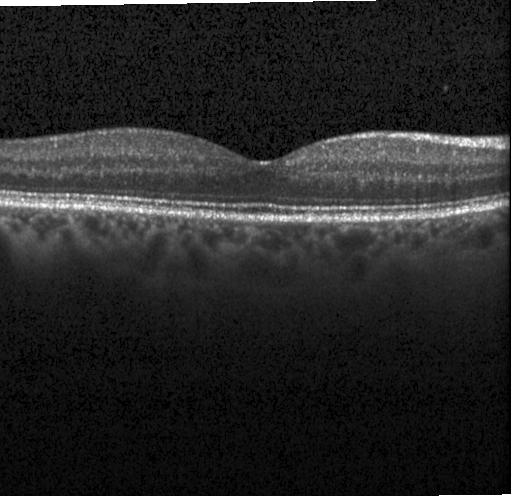

Macular OCT demonstrating no CNV, DME, or drusen.